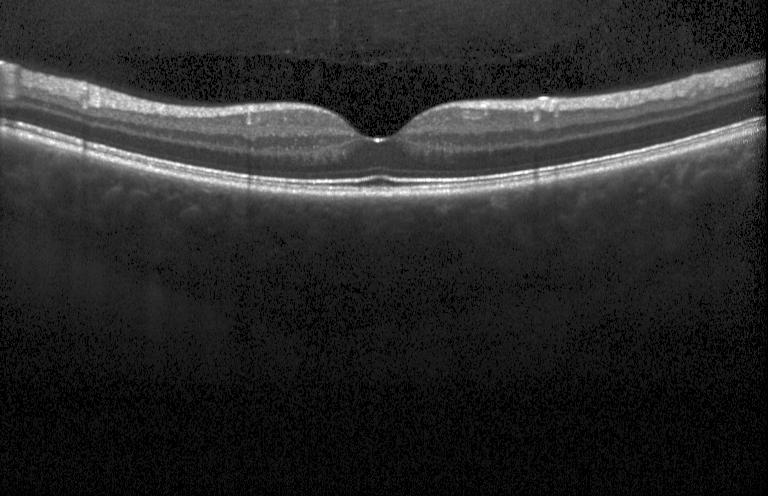
Retinal OCT cross-section, macular scan, spectral-domain OCT, acquired on a Heidelberg Spectralis — Dx: no evidence of CNV, DME, or drusen.